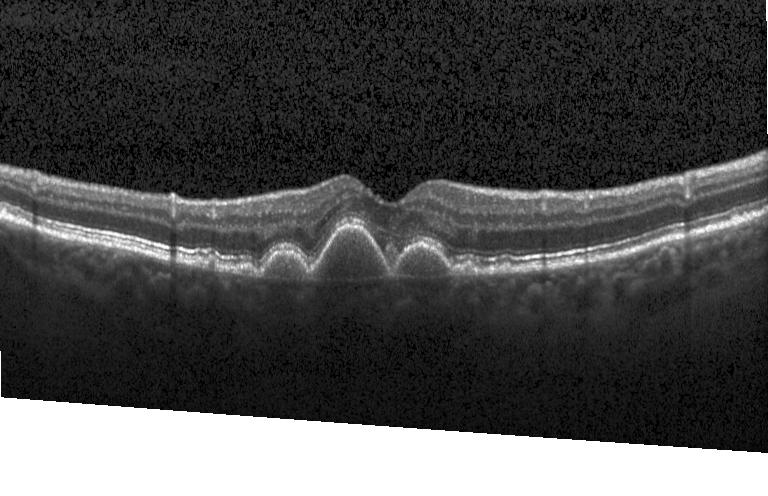

Retinal OCT cross-section. Heidelberg Spectralis OCT system. Centered on the fovea. Spectral-domain optical coherence tomography — Macular OCT: a choroidal neovascular membrane.